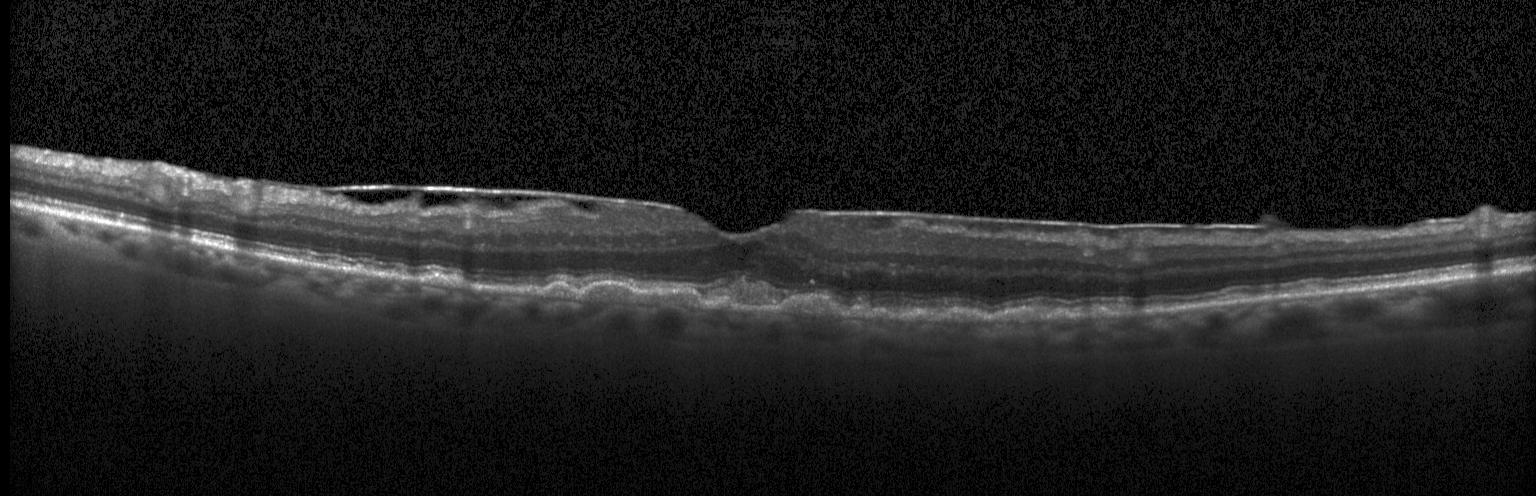

Fovea-centered. Retinal OCT B-scan
Diagnosis: sub-RPE drusenoid deposits.